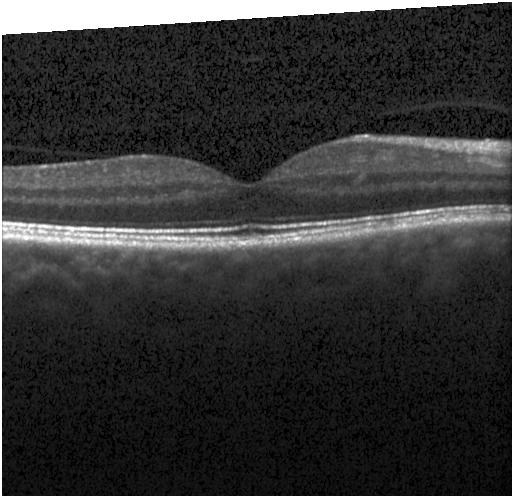
Heidelberg Spectralis OCT system. Spectral-domain optical coherence tomography. Optical coherence tomography B-scan. Centered on the fovea.
The scan shows no choroidal neovascularization, no diabetic macular edema, and no drusen.